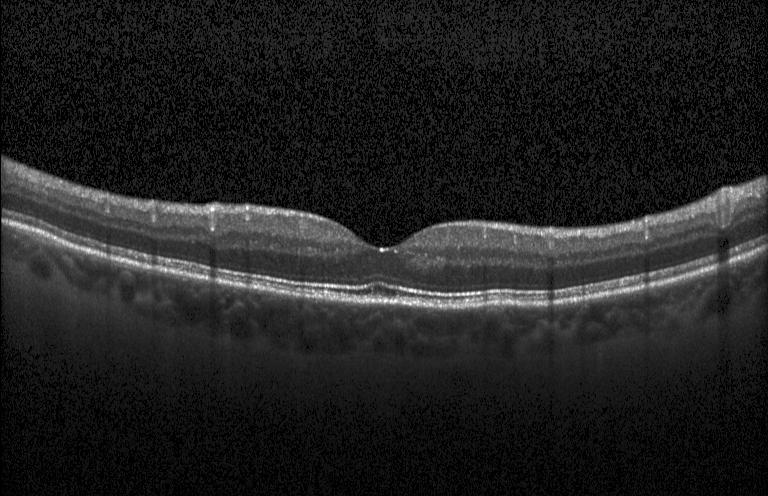 OCT finding: no evidence of choroidal neovascularization, diabetic macular edema, or drusen.